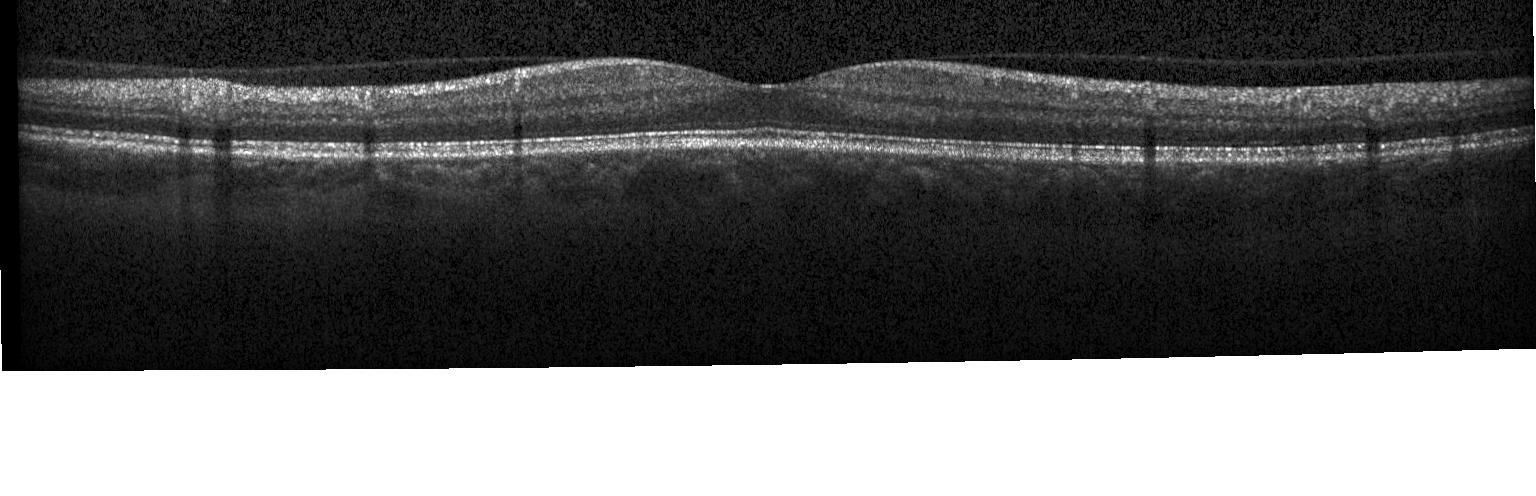
OCT line scan
Impression: no CNV, no DME, and no drusen.